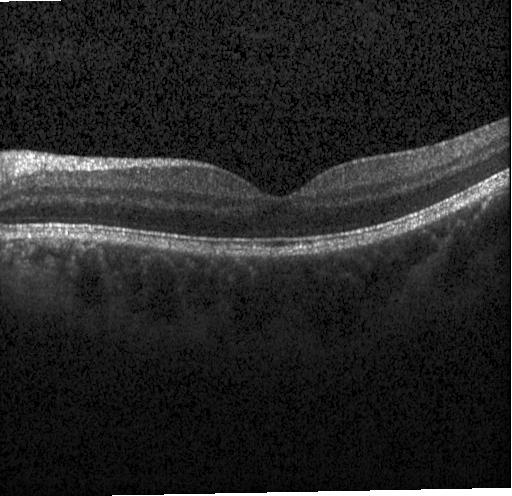

Optical coherence tomography B-scan · SD-OCT.
Assessment: neither choroidal neovascularization, diabetic macular edema, nor drusen.